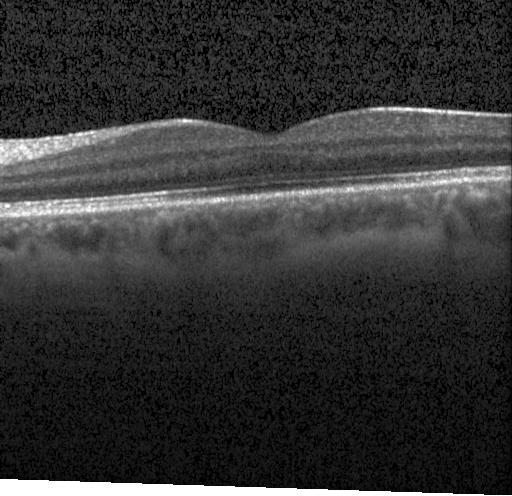 Retinal OCT B-scan.
No choroidal neovascularization, no diabetic macular edema, and no drusen.